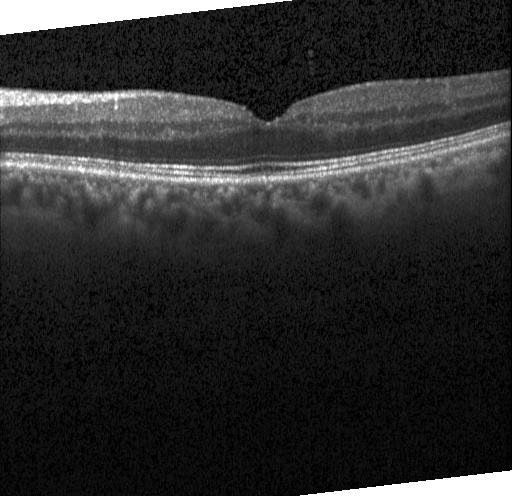
Through the macula, OCT B-scan, SD-OCT, acquired on a Heidelberg Spectralis. The scan shows neither choroidal neovascularization, diabetic macular edema, nor drusen.